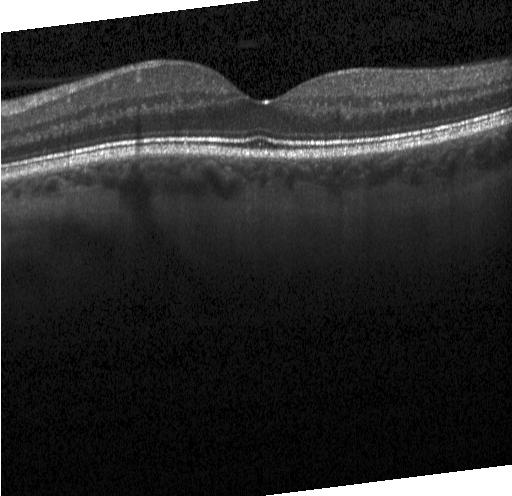

Diagnosis: no choroidal neovascularization, diabetic macular edema, or drusen.